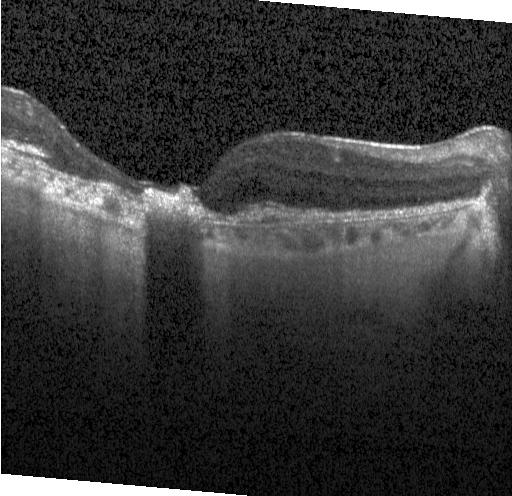 Optical coherence tomography scan; spectral-domain optical coherence tomography — Impression: a choroidal neovascular membrane.